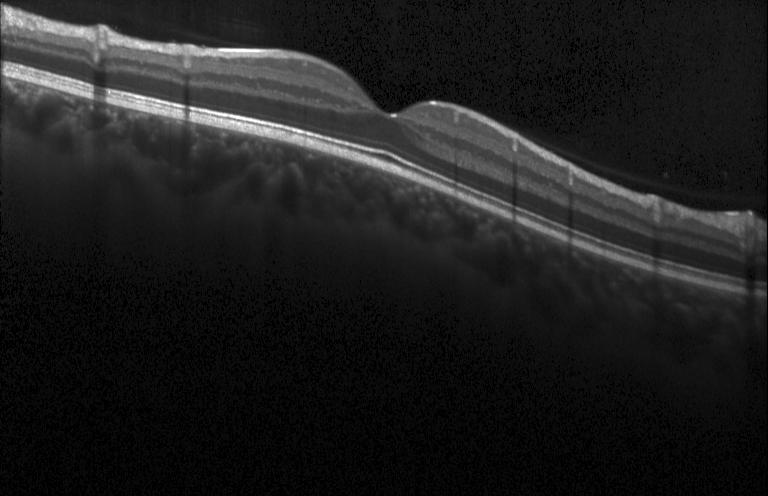 Impression: neither choroidal neovascularization, diabetic macular edema, nor drusen.